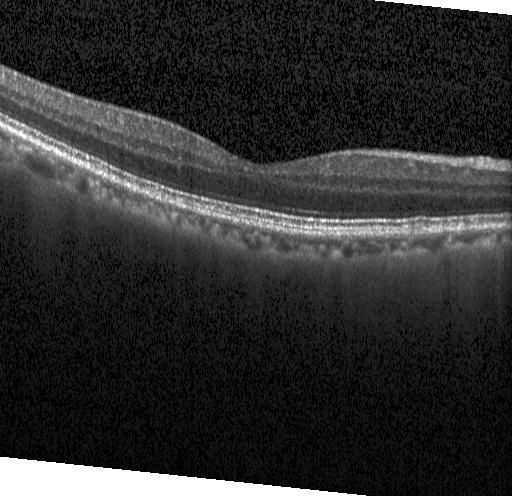
OCT line scan — This B-scan demonstrates neither choroidal neovascularization, diabetic macular edema, nor drusen.